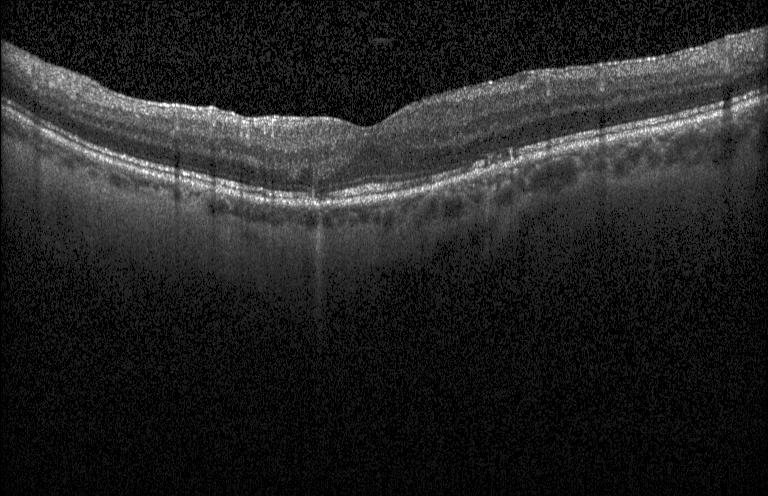 Dx: no evidence of choroidal neovascularization, diabetic macular edema, or drusen.